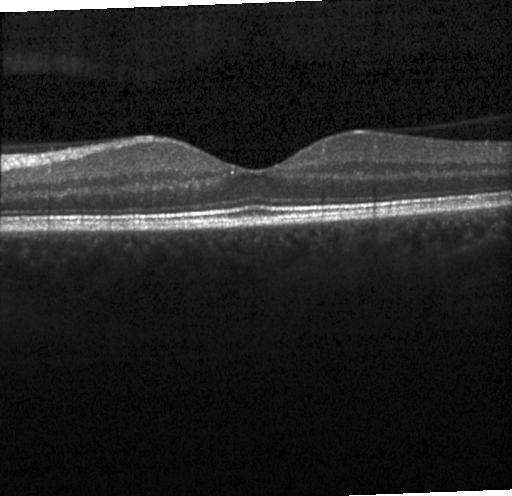
OCT B-scan showing no evidence of CNV, DME, or drusen.